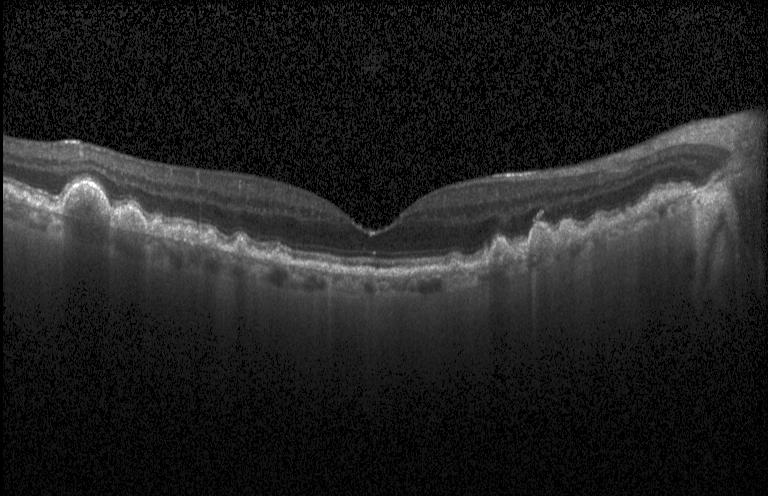

OCT finding: drusen.